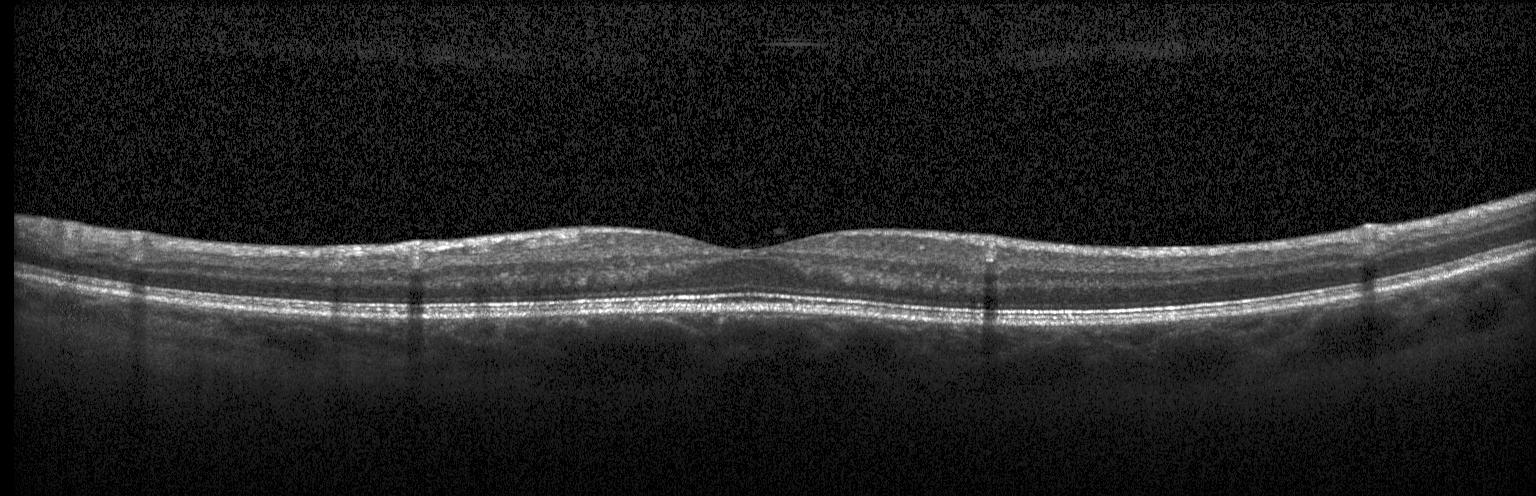
OCT line scan. Impression: neither CNV, DME, nor drusen.